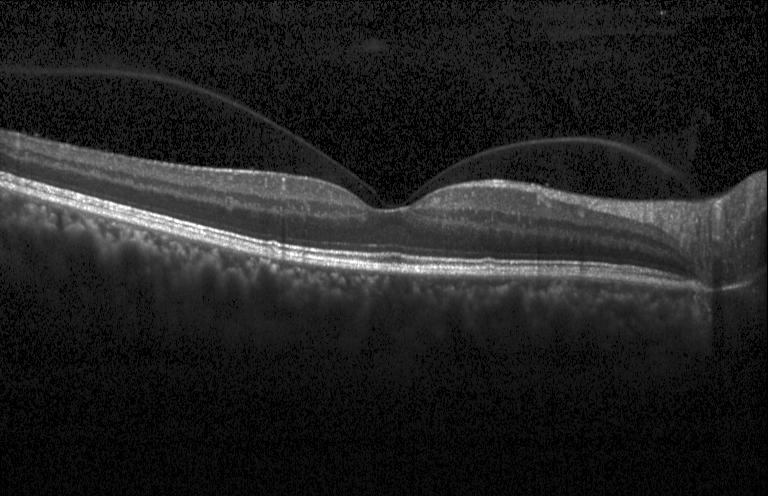 OCT line scan. The scan shows neither choroidal neovascularization, diabetic macular edema, nor drusen.